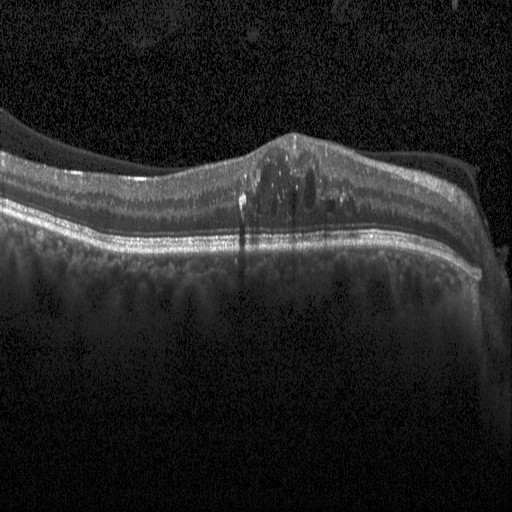 Diagnosis: diabetic macular edema.